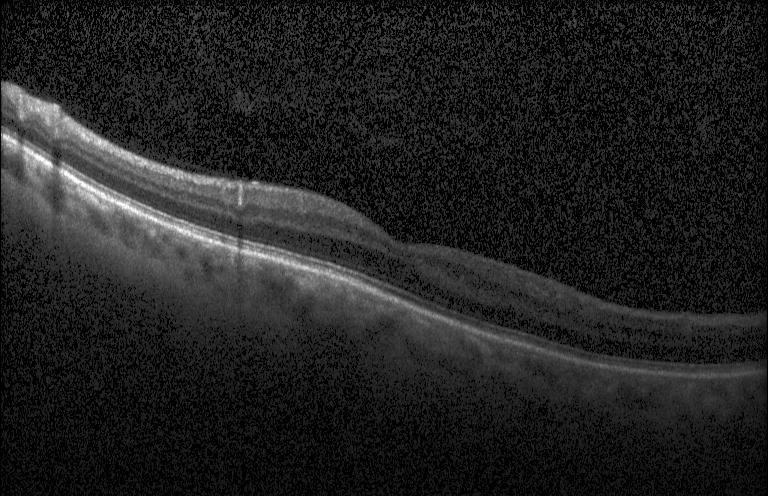
Optical coherence tomography B-scan
Macular OCT: no choroidal neovascularization, diabetic macular edema, or drusen.